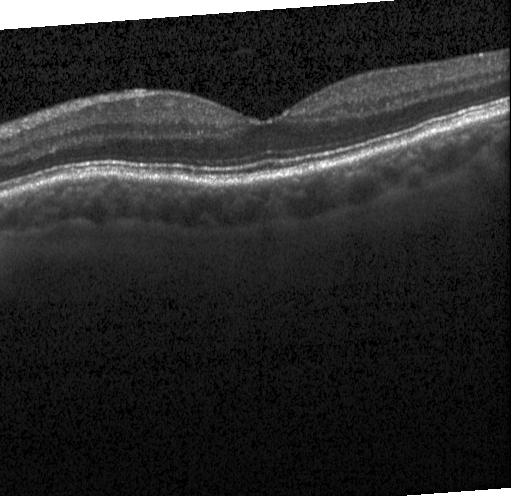 Retinal OCT B-scan. Finding: no CNV, DME, or drusen.